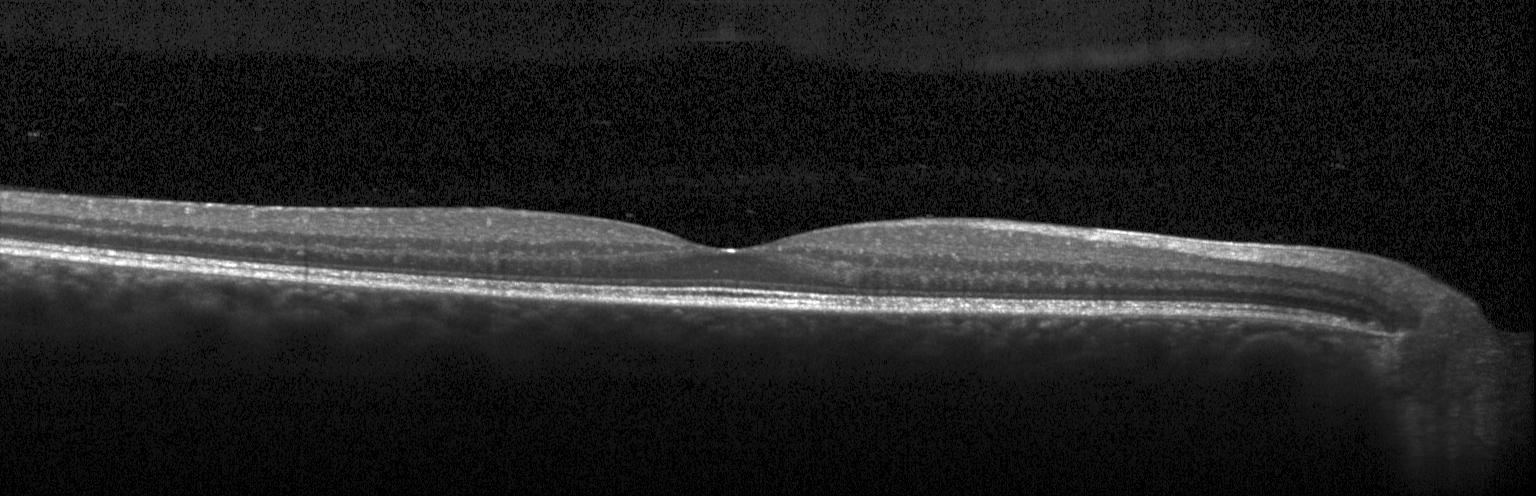 OCT line scan. Dx: no choroidal neovascularization, diabetic macular edema, or drusen.